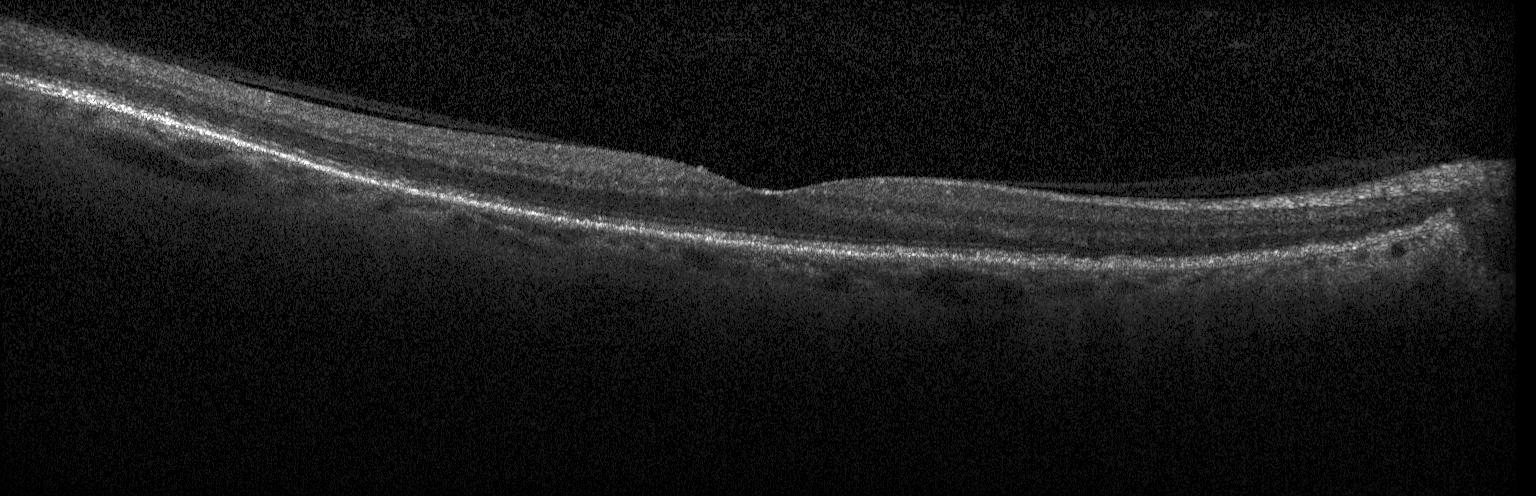 Macular OCT: no choroidal neovascularization, diabetic macular edema, or drusen.